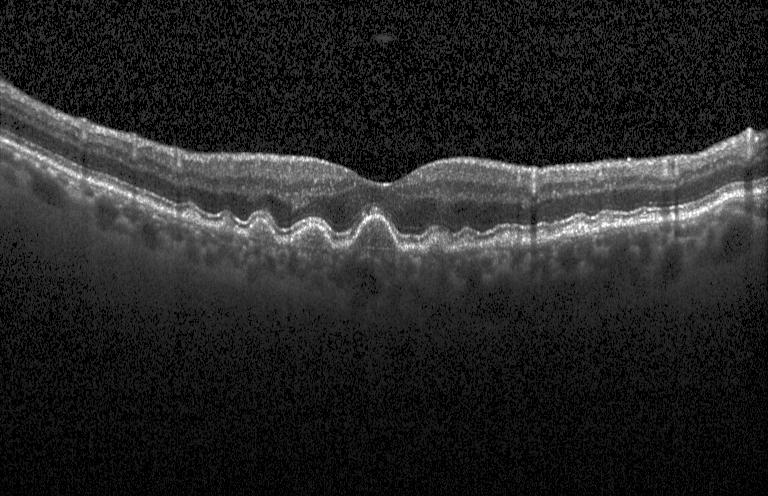 OCT B-scan showing sub-RPE drusenoid deposits.